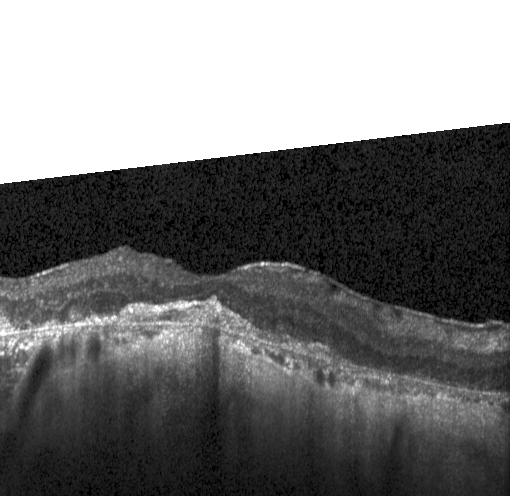
Spectral-domain OCT; through the macula; optical coherence tomography scan
This B-scan demonstrates choroidal neovascularization (CNV).